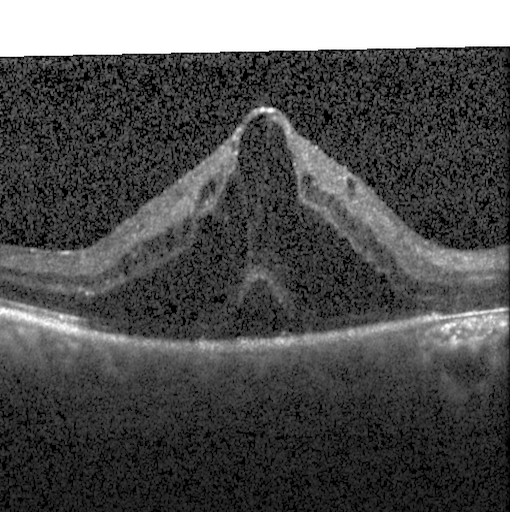 Retinal OCT B-scan; spectral-domain OCT; centered on the fovea; instrument: Heidelberg Spectralis
This B-scan demonstrates diabetic macular edema (DME).